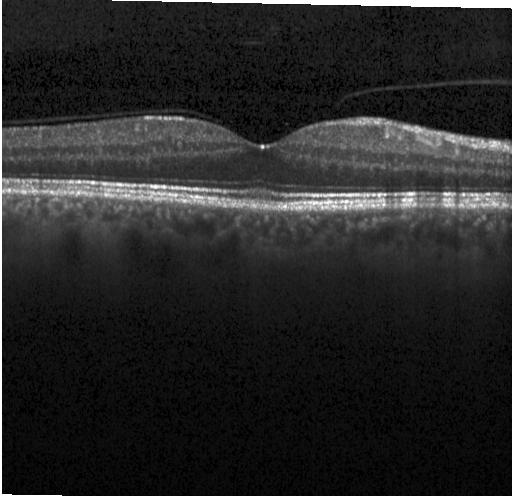

Instrument: Heidelberg Spectralis · retinal OCT B-scan · fovea-centered · SD-OCT.
Impression: neither choroidal neovascularization, diabetic macular edema, nor drusen.